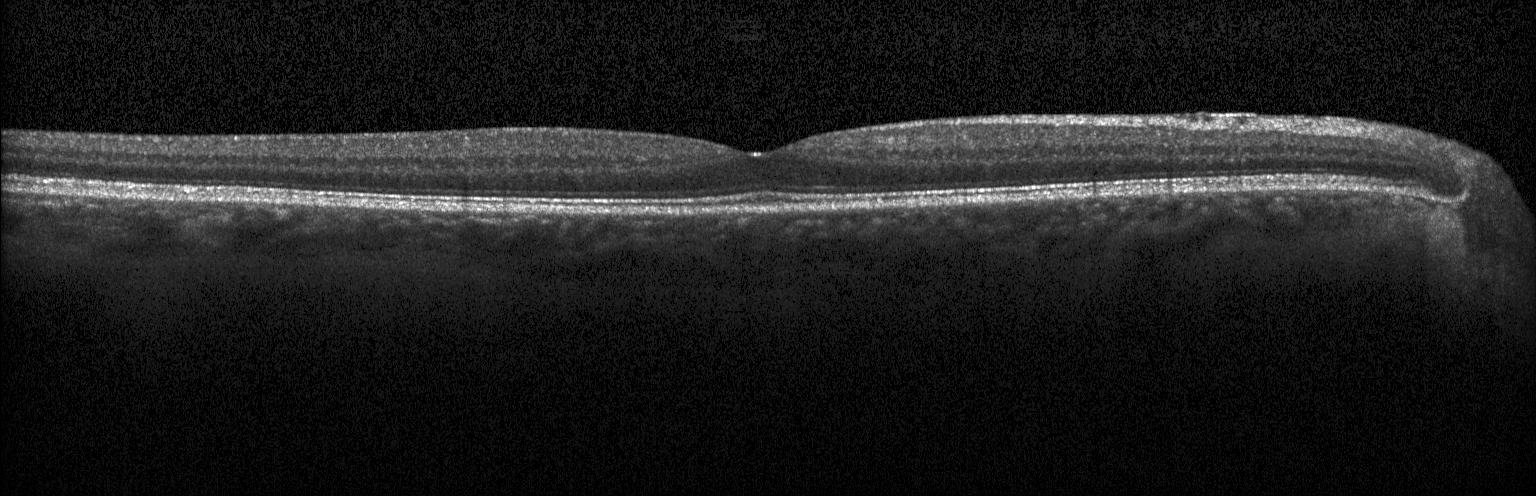

Instrument: Heidelberg Spectralis · optical coherence tomography B-scan
Diagnosis: no choroidal neovascularization, diabetic macular edema, or drusen.